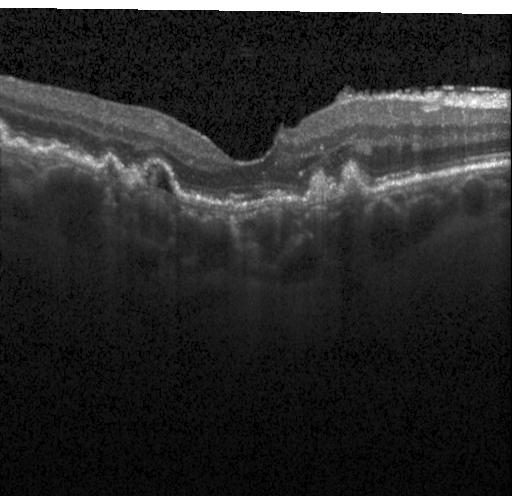 Retinal OCT cross-section. Centered on the fovea. Heidelberg Spectralis OCT system
OCT finding: choroidal neovascularization (CNV).